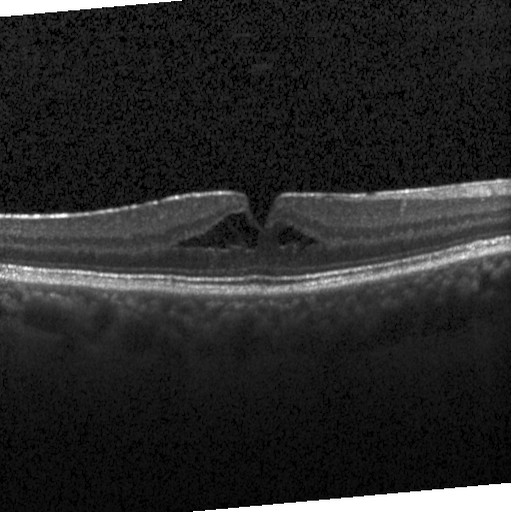 Spectral-domain OCT, retinal OCT B-scan, Heidelberg Spectralis OCT system
This B-scan demonstrates diabetic macular edema.